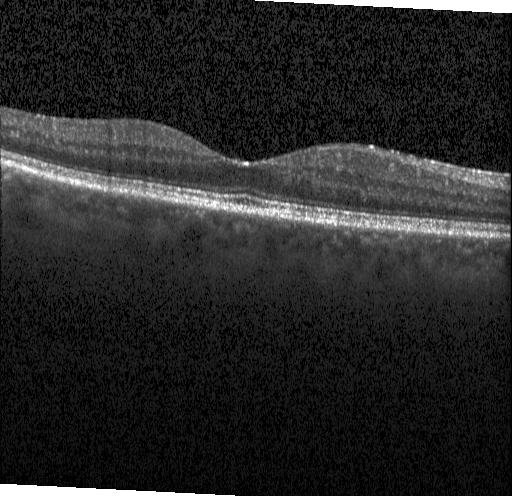
Spectral-domain optical coherence tomography. OCT line scan — Diagnosis: no choroidal neovascularization, no diabetic macular edema, and no drusen.